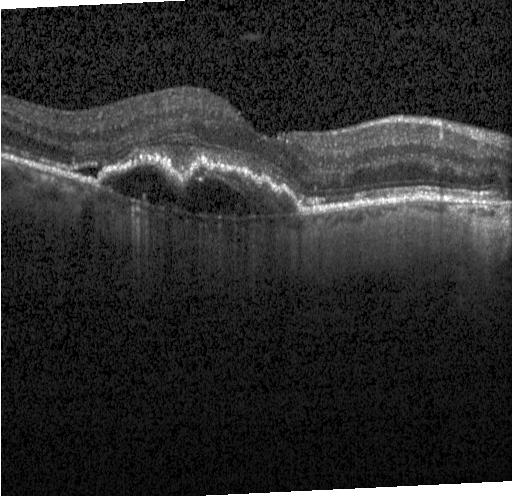

Optical coherence tomography B-scan; spectral-domain OCT. OCT finding: a choroidal neovascular membrane.